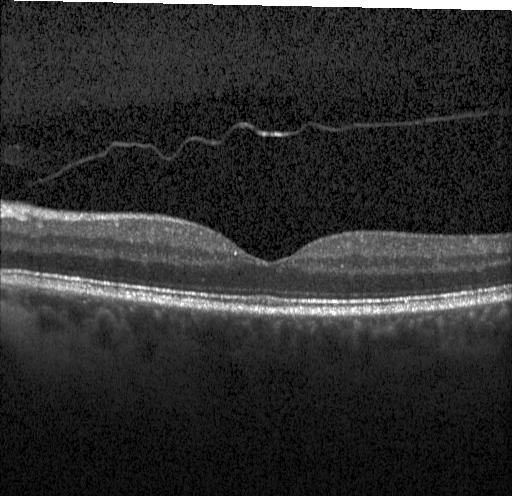

OCT finding: neither choroidal neovascularization, diabetic macular edema, nor drusen.